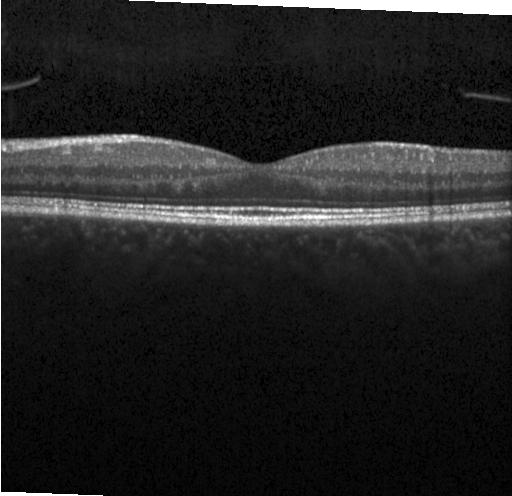

Finding: neither CNV, DME, nor drusen.